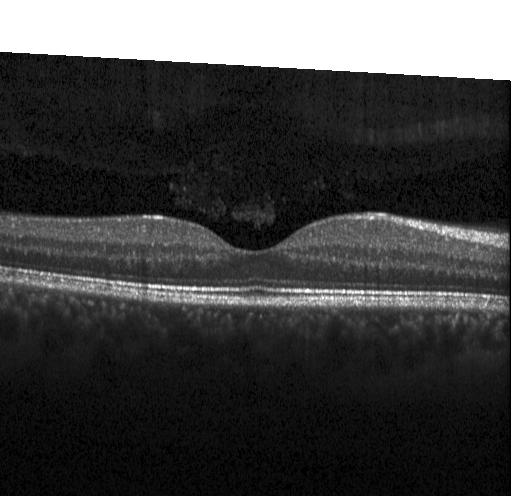
Finding: no choroidal neovascularization, diabetic macular edema, or drusen.